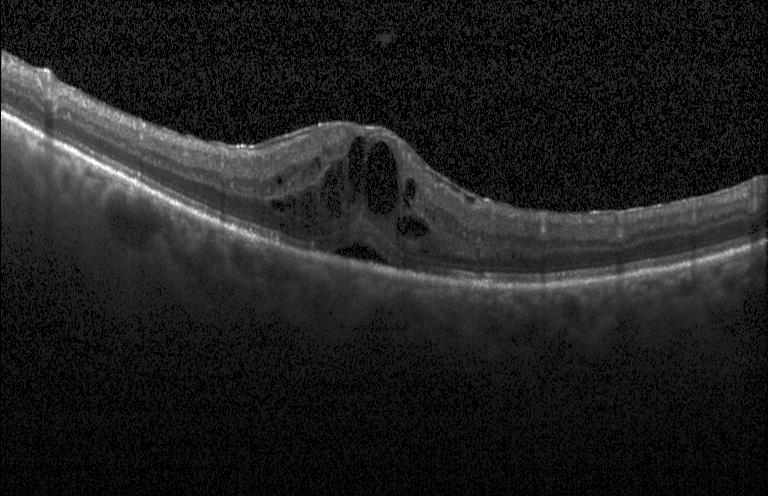
Acquired on a Heidelberg Spectralis; spectral-domain optical coherence tomography; horizontal scan through the fovea; retinal OCT cross-section. Impression: diabetic macular edema (DME).